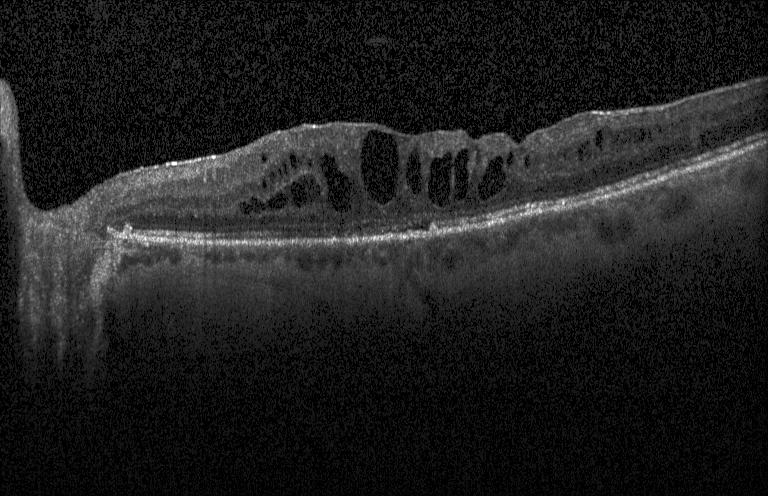 OCT finding: DME.